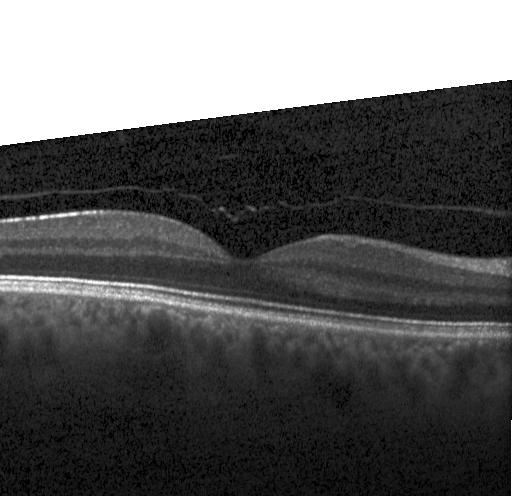

Dx: no choroidal neovascularization, no diabetic macular edema, and no drusen.